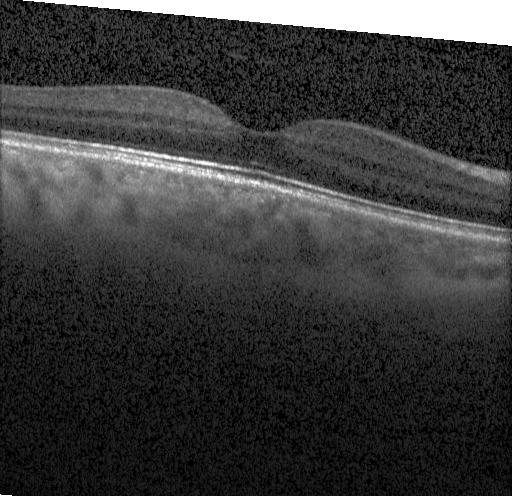
Acquired on a Heidelberg Spectralis. Retinal OCT cross-section
Finding: no CNV, DME, or drusen.